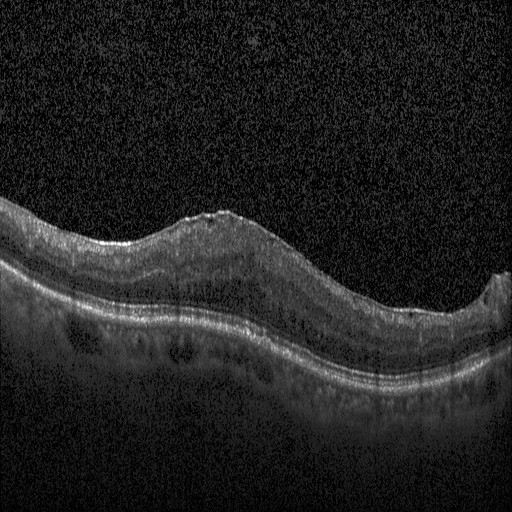 OCT B-scan. Instrument: Heidelberg Spectralis. Through the macula
Finding: DME.